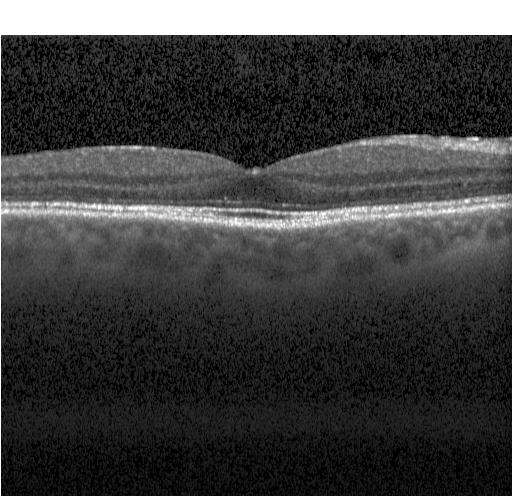

Instrument: Heidelberg Spectralis, spectral-domain OCT, retinal OCT B-scan — Diagnosis: no evidence of choroidal neovascularization, diabetic macular edema, or drusen.